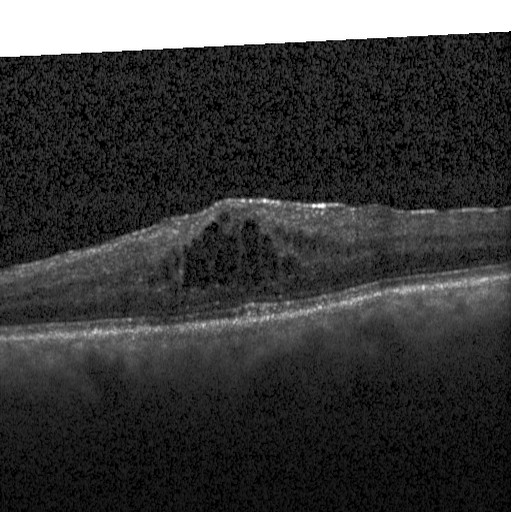

Retinal OCT B-scan. Spectral-domain optical coherence tomography. Heidelberg Spectralis. Horizontal scan through the fovea. Finding: diabetic macular edema.